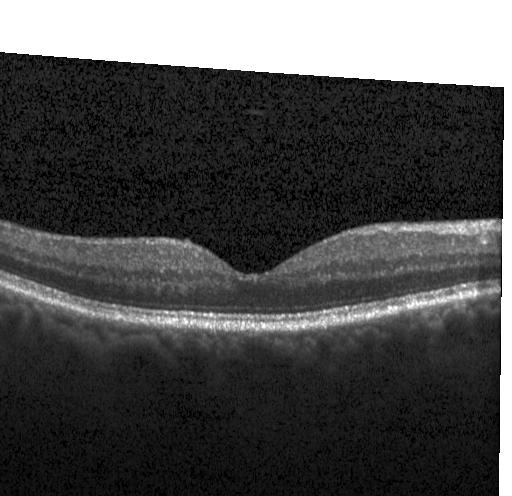

Finding: no evidence of choroidal neovascularization, diabetic macular edema, or drusen.